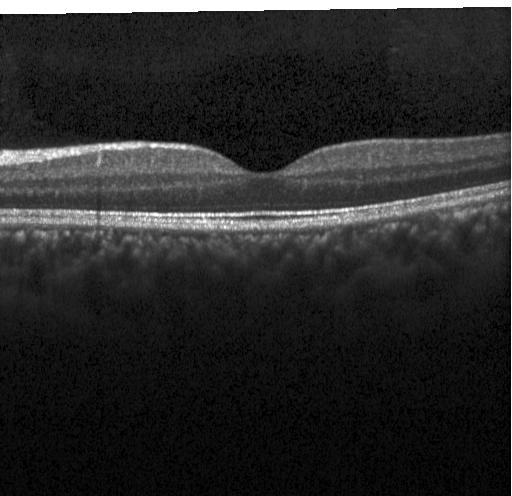
Assessment: no choroidal neovascularization, diabetic macular edema, or drusen.